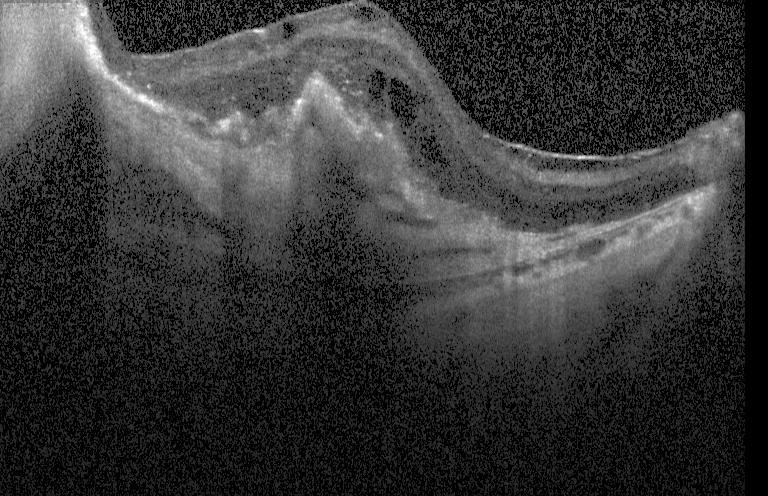
Choroidal neovascularization (CNV).